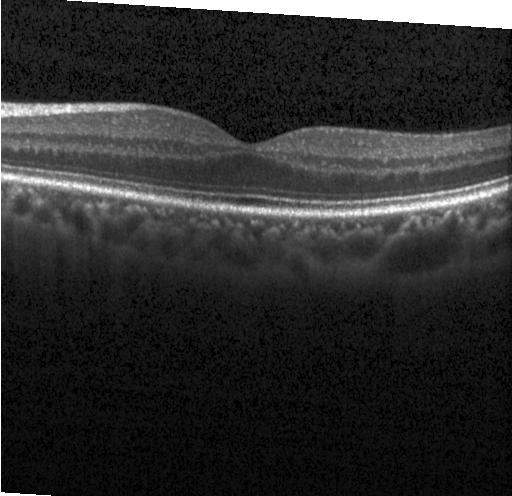
OCT B-scan
Dx: no evidence of choroidal neovascularization, diabetic macular edema, or drusen.